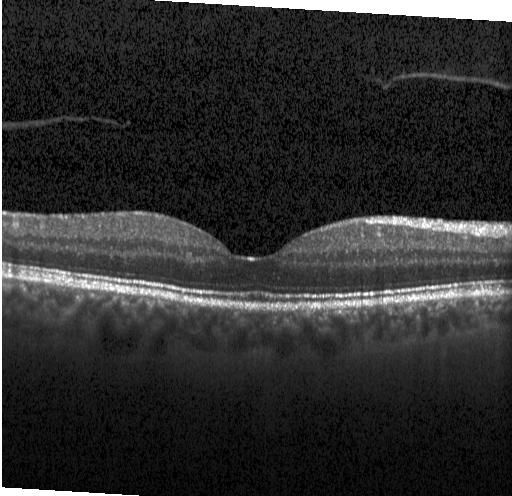 Spectral-domain OCT B-scan: no CNV, DME, or drusen.